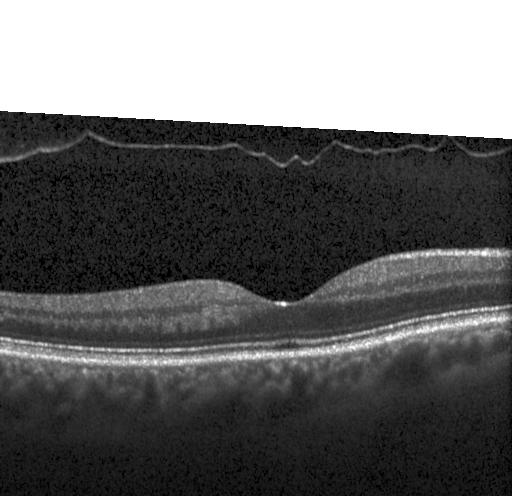
OCT B-scan
Finding: no CNV, no DME, and no drusen.